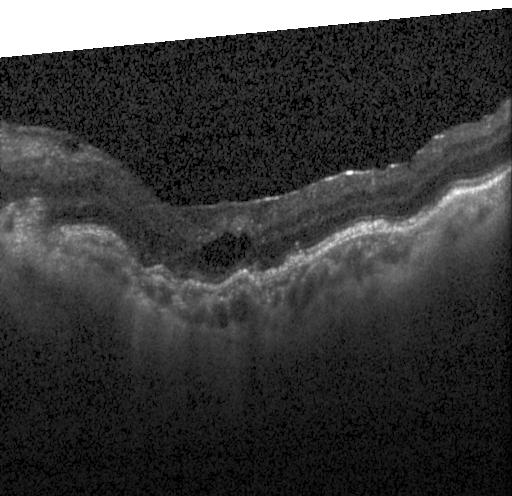
OCT B-scan showing a choroidal neovascular membrane.